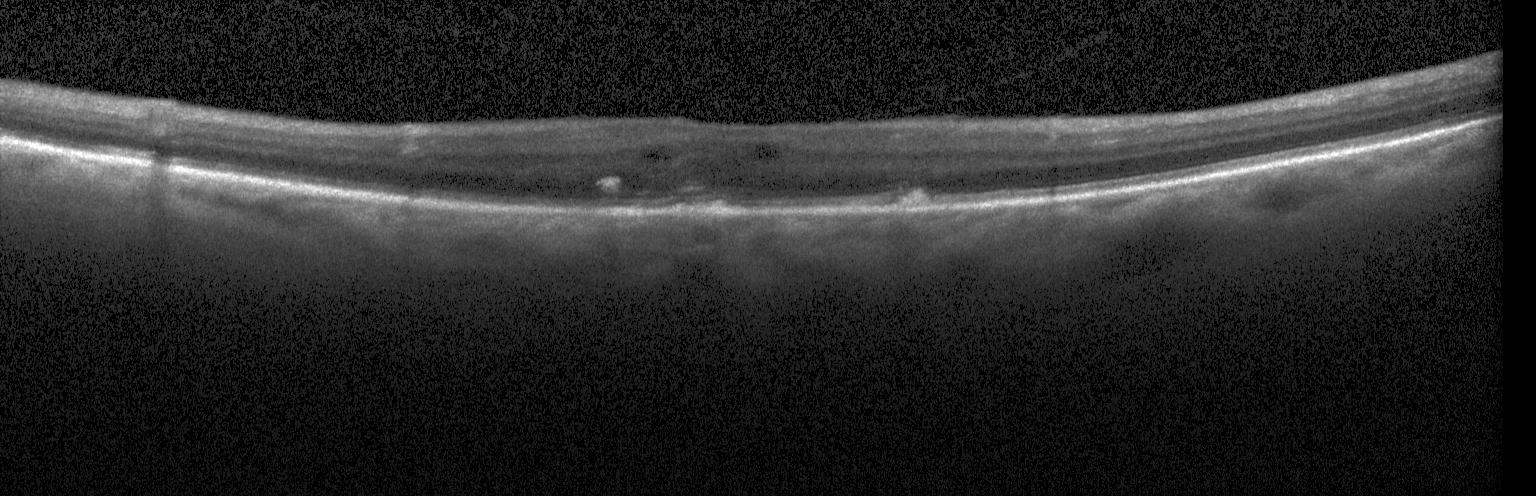 Diagnosis: diabetic macular edema (DME).